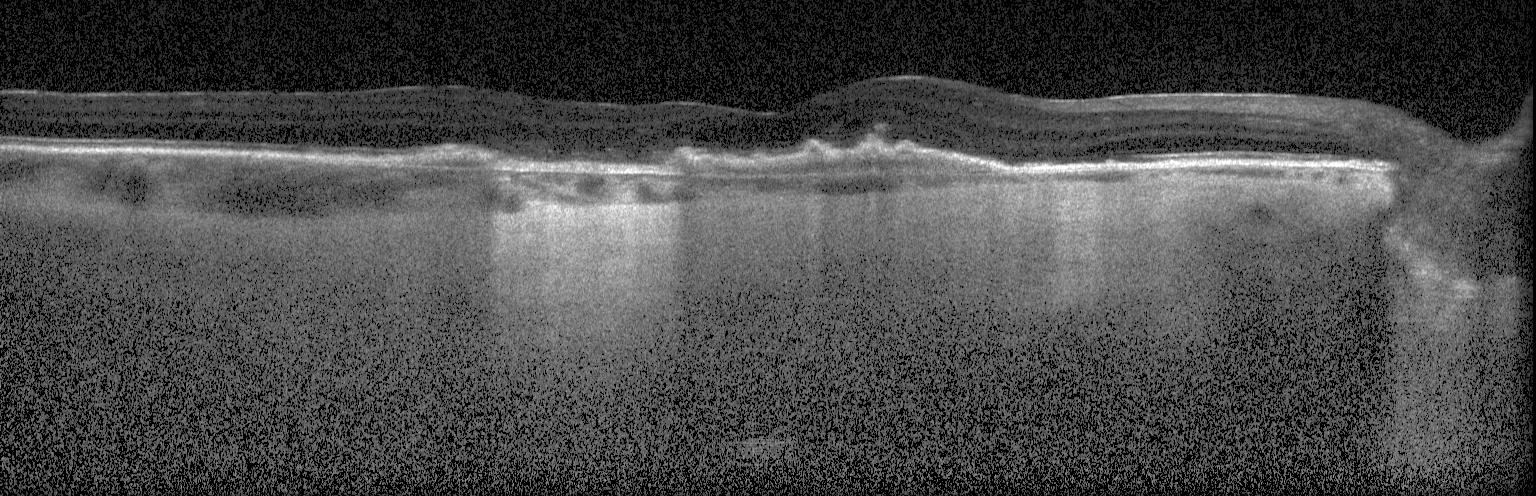
Macular scan, retinal OCT cross-section, spectral-domain optical coherence tomography, instrument: Heidelberg Spectralis
Assessment: choroidal neovascularization.